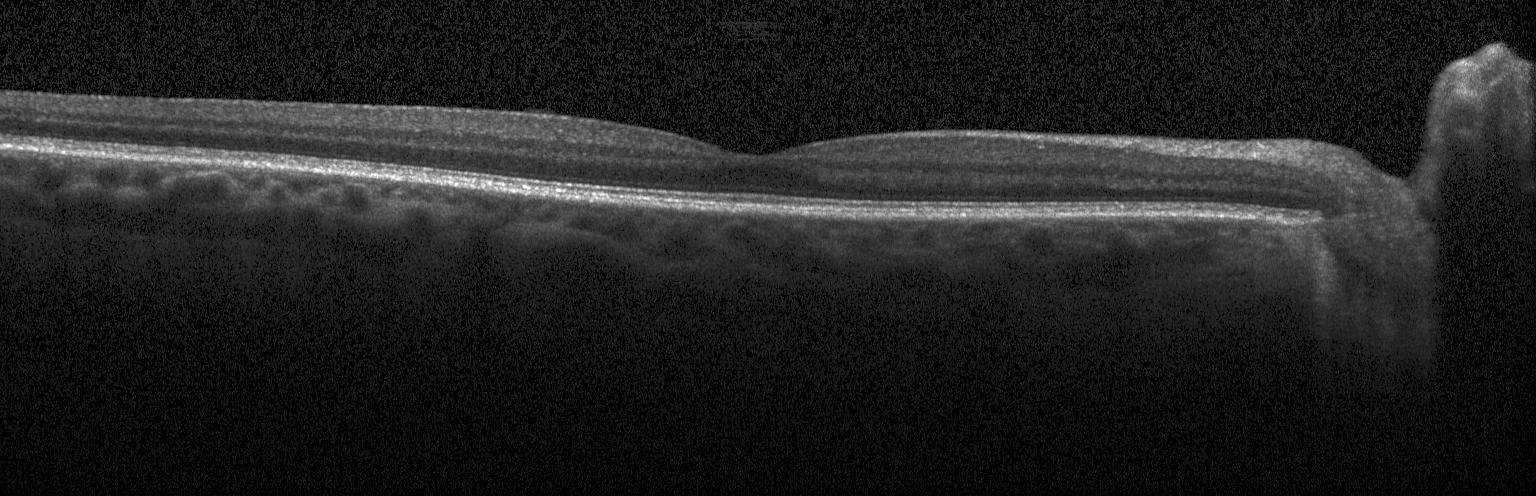 Retinal OCT cross-section showing no choroidal neovascularization, no diabetic macular edema, and no drusen.